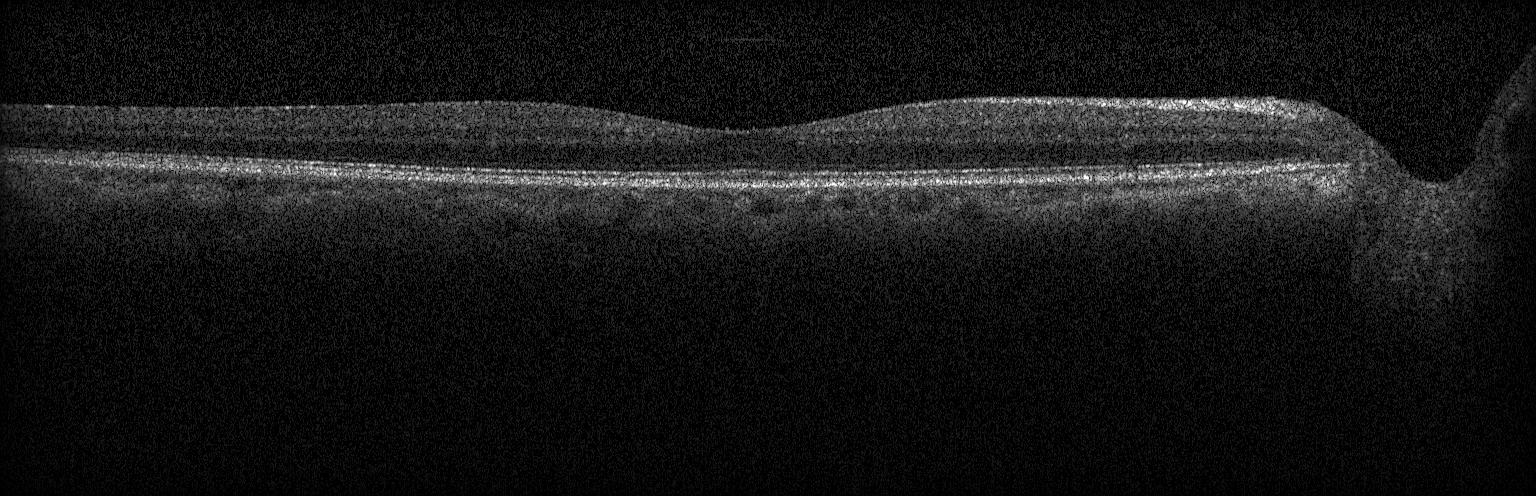

Heidelberg Spectralis, fovea-centered, spectral-domain OCT, OCT B-scan.
Macular OCT: no CNV, no DME, and no drusen.